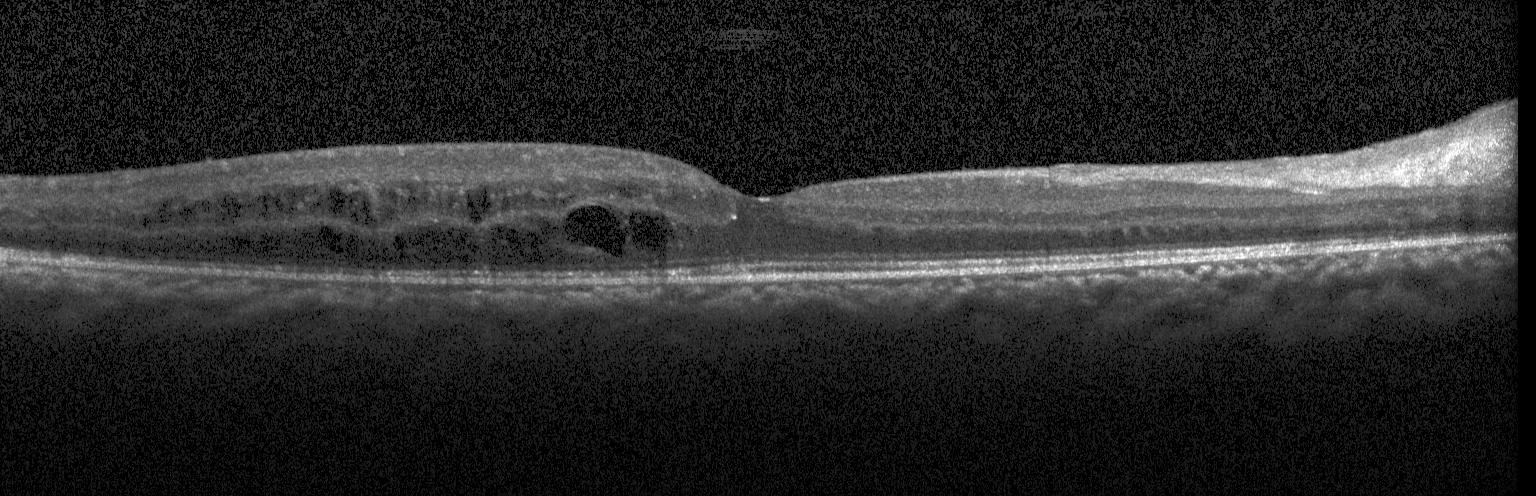
Dx: diabetic macular edema.